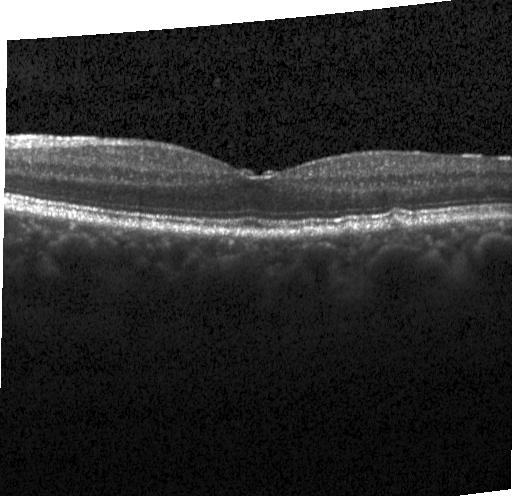
Dx: multiple drusen.